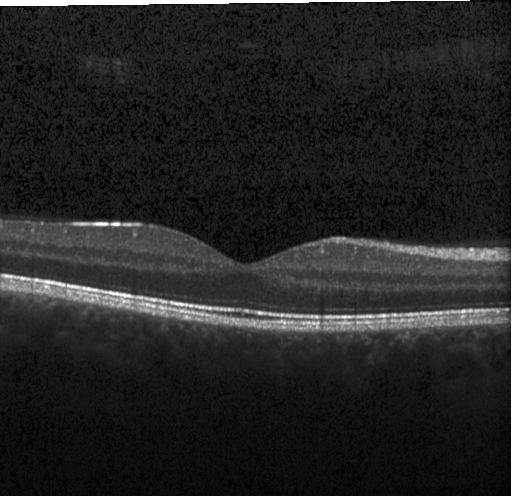

Horizontal scan through the fovea. Retinal OCT cross-section. Heidelberg Spectralis. Spectral-domain optical coherence tomography — OCT finding: no CNV, no DME, and no drusen.